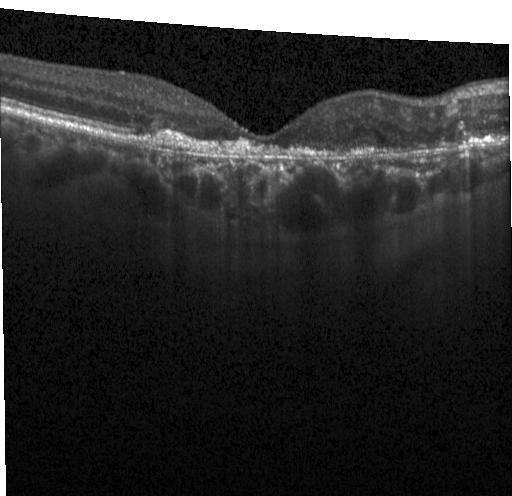 Centered on the fovea · SD-OCT · OCT line scan.
The scan shows CNV.